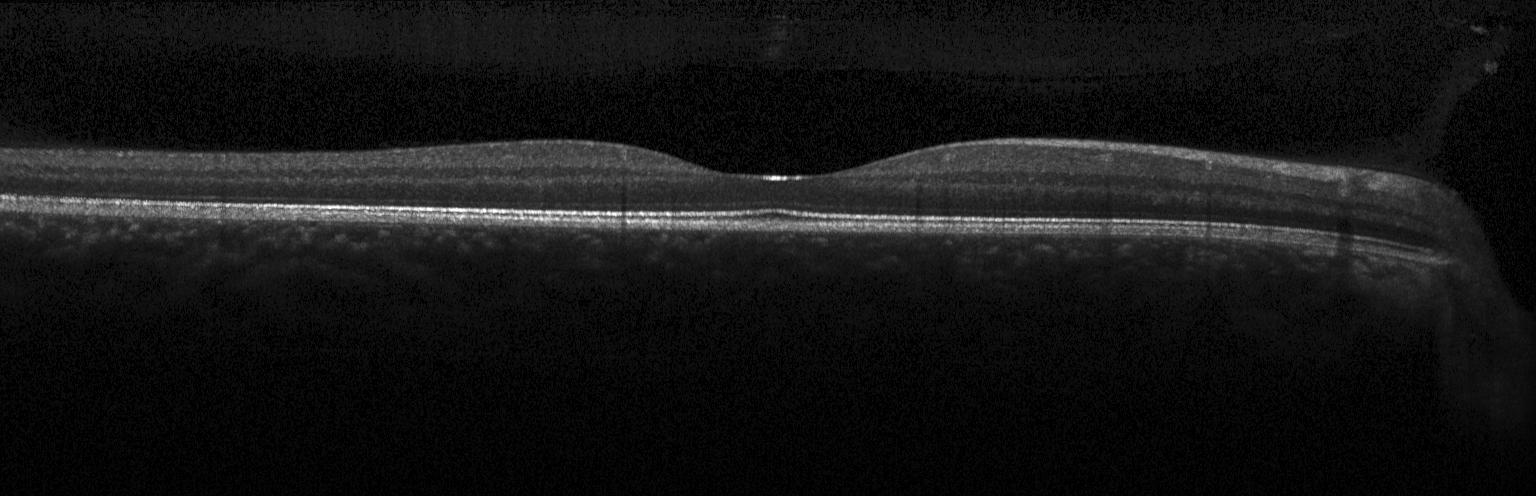
Horizontal scan through the fovea, spectral-domain optical coherence tomography, retinal OCT B-scan.
Assessment: neither CNV, DME, nor drusen.